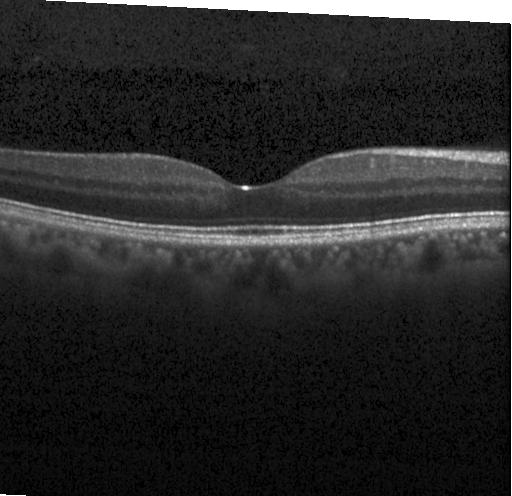 Spectral-domain optical coherence tomography, retinal OCT B-scan, centered on the fovea — This B-scan demonstrates neither choroidal neovascularization, diabetic macular edema, nor drusen.